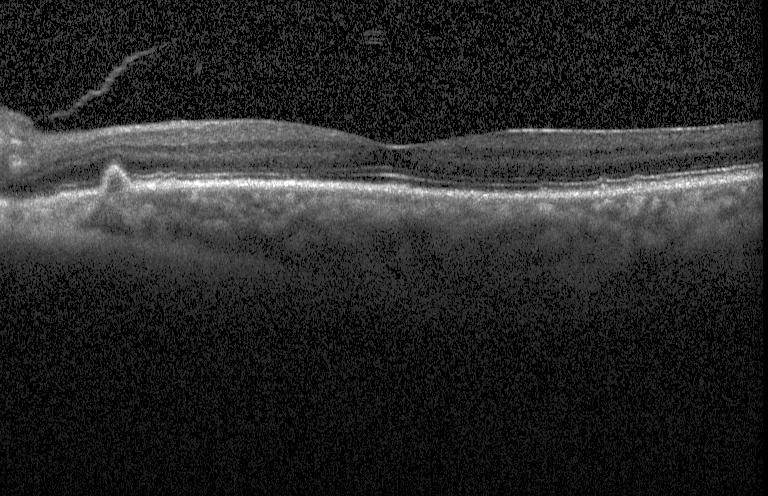

OCT finding: drusen.